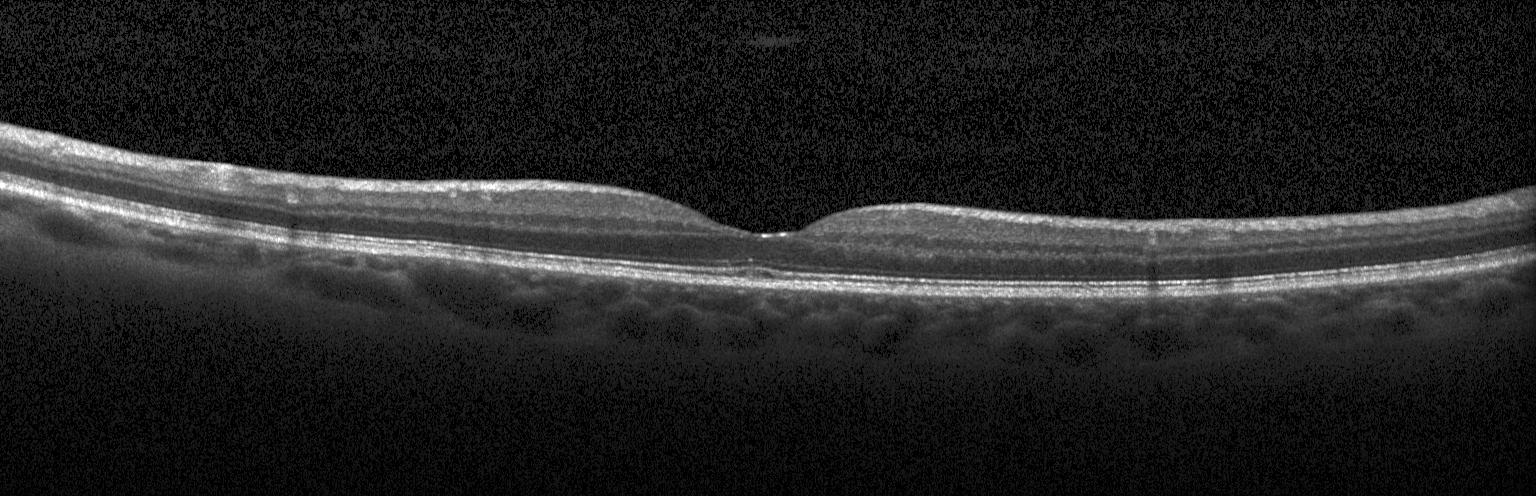
OCT B-scan showing no choroidal neovascularization, diabetic macular edema, or drusen.